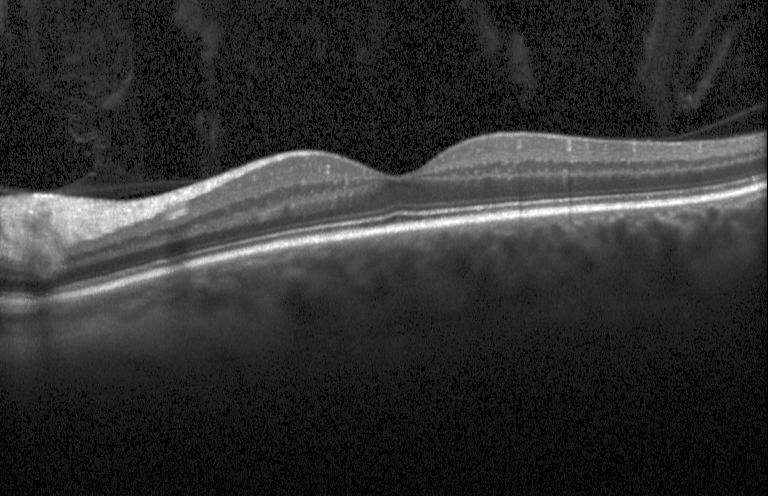 Through the macula. Instrument: Heidelberg Spectralis. Retinal OCT cross-section
Impression: no choroidal neovascularization, diabetic macular edema, or drusen.